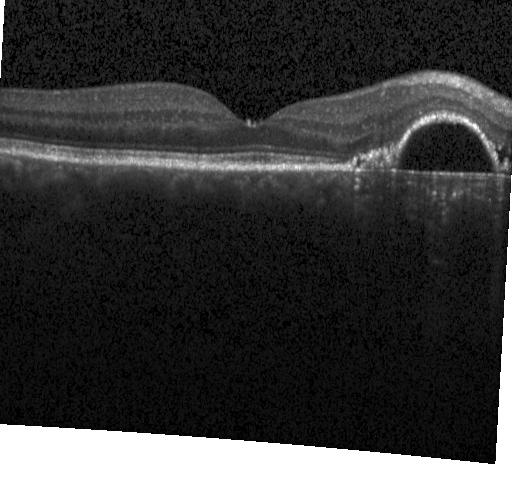

OCT line scan. Assessment: choroidal neovascularization (CNV).